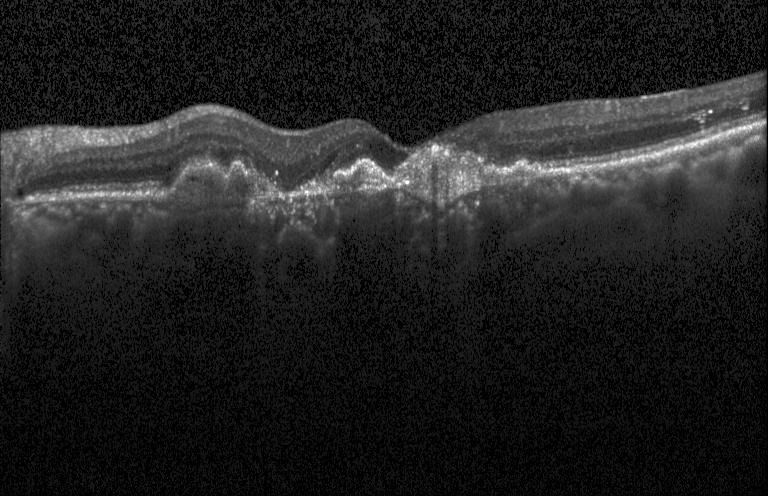 Retinal OCT B-scan, Heidelberg Spectralis — Assessment: choroidal neovascularization (CNV).